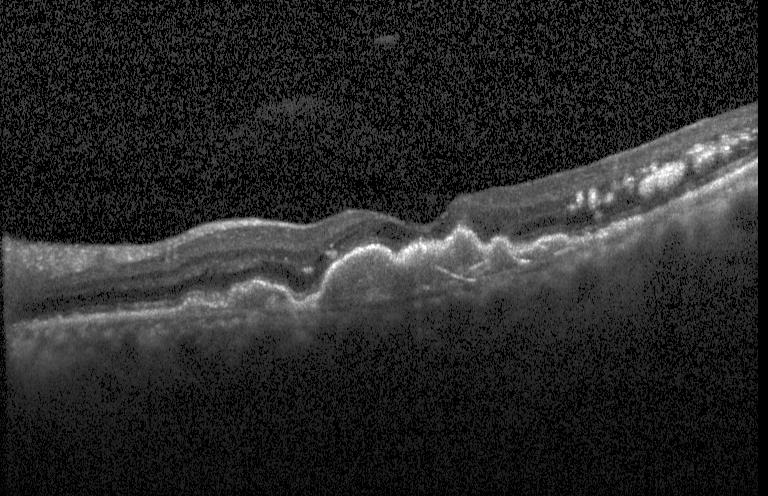 Optical coherence tomography B-scan, centered on the fovea.
Dx: a choroidal neovascular membrane.